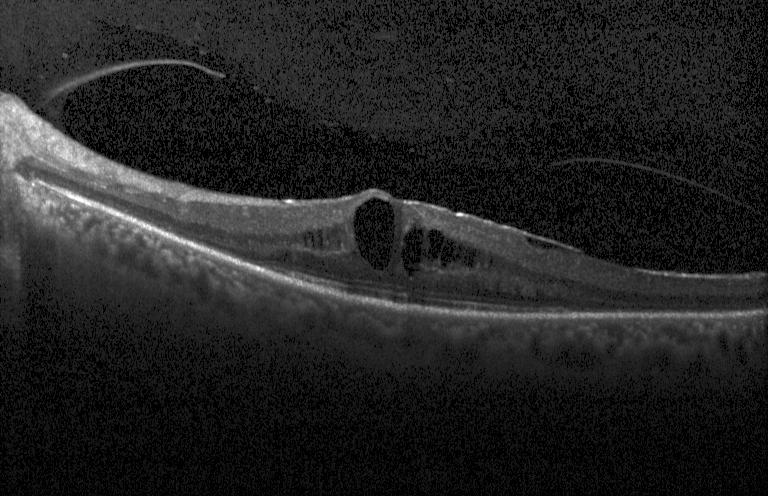

Through the macula · spectral-domain OCT · acquired on a Heidelberg Spectralis · retinal OCT cross-section
Diagnosis: diabetic macular edema (DME).